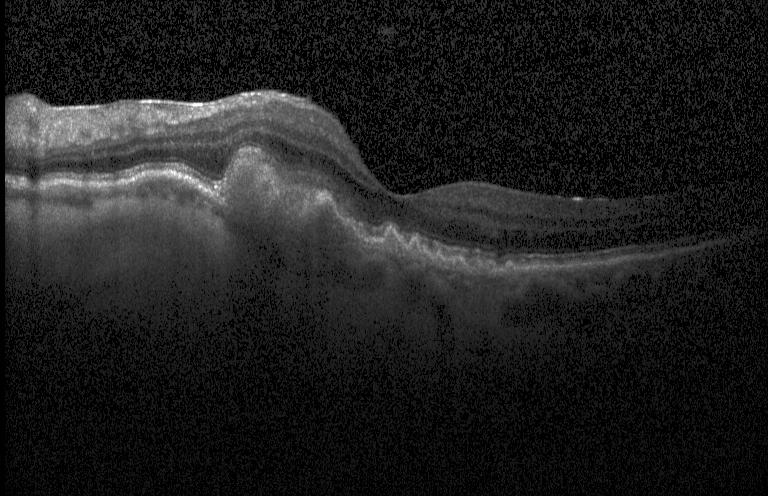 Optical coherence tomography scan, instrument: Heidelberg Spectralis.
Macular OCT: a choroidal neovascular membrane.